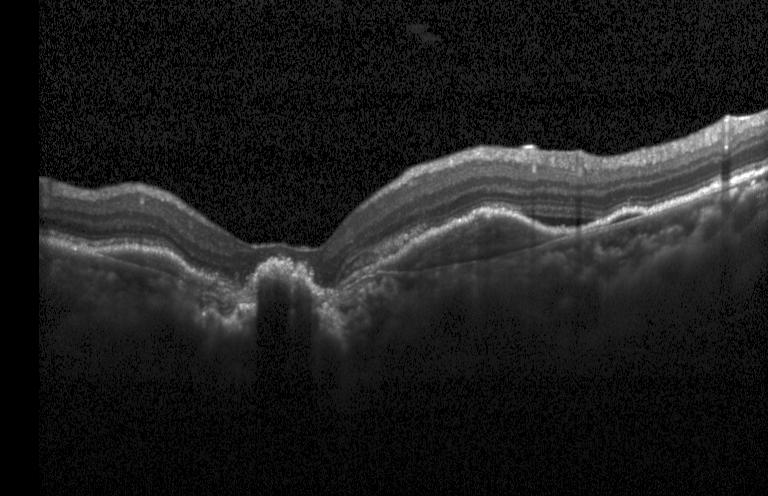
OCT finding: choroidal neovascularization.